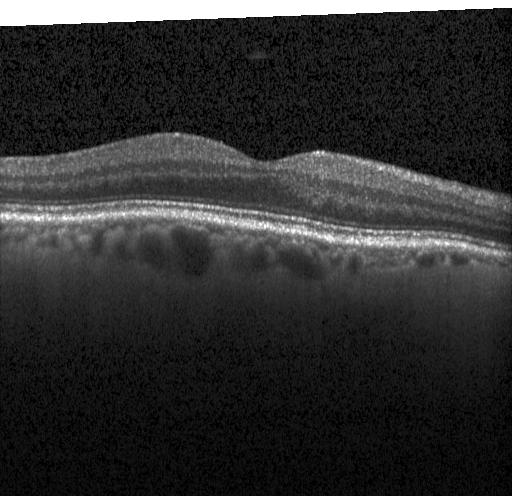

Assessment: neither choroidal neovascularization, diabetic macular edema, nor drusen.